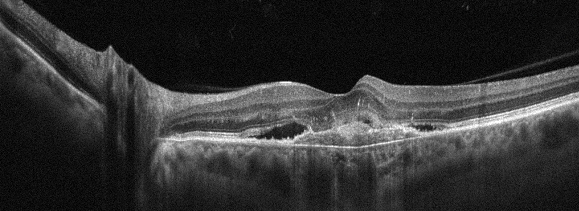

OCT B-scan · acquired on an Optovue Avanti RTVue XR · oculus sinister
The scan shows AMD.